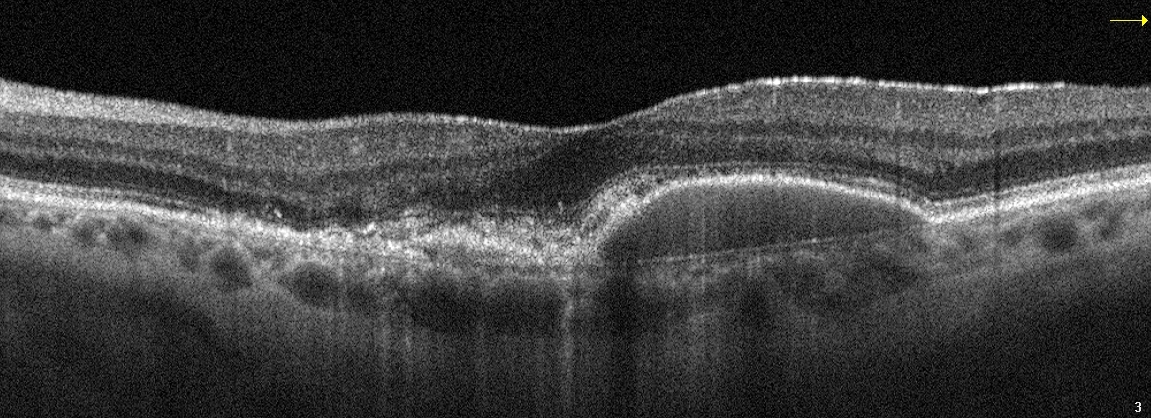
Age-related macular degeneration (AMD).